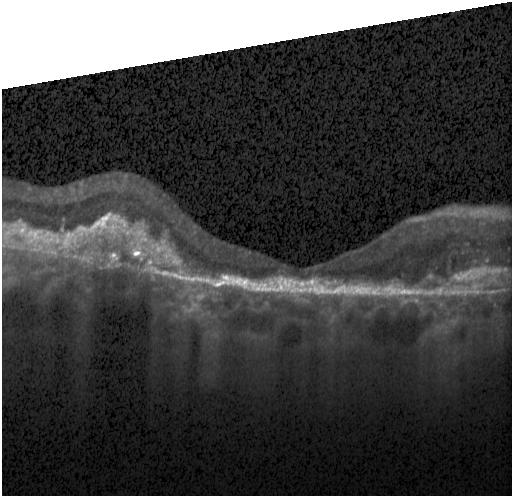 OCT finding: a choroidal neovascular membrane.